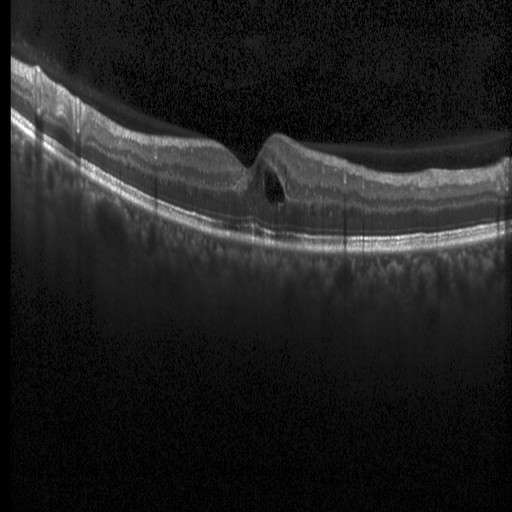 Heidelberg Spectralis OCT system; OCT line scan
Diagnosis: DME.